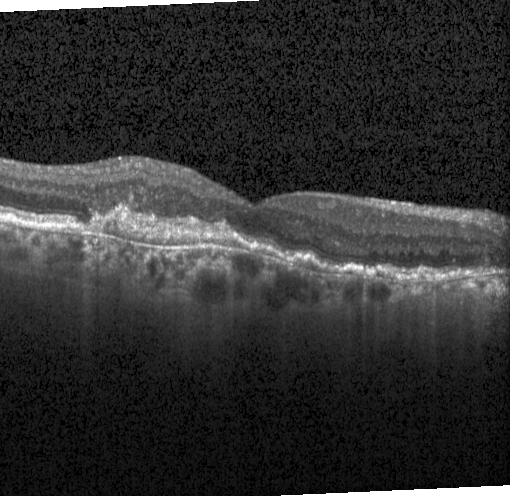
Impression: a choroidal neovascular membrane.